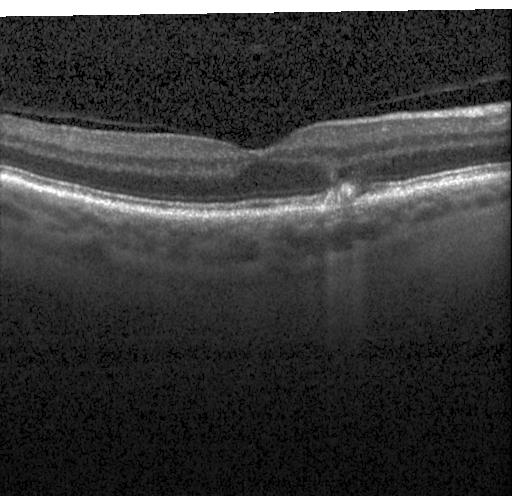 Optical coherence tomography scan. Heidelberg Spectralis. SD-OCT. Fovea-centered. Diagnosis: drusen.